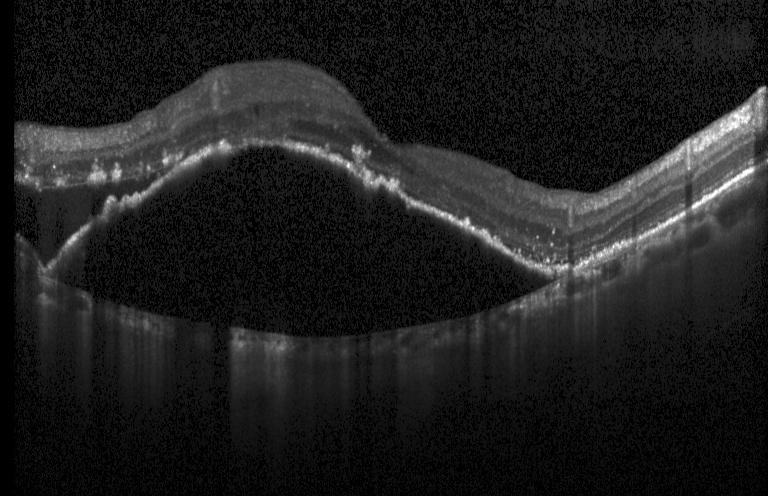
Optical coherence tomography B-scan. Acquired on a Heidelberg Spectralis.
Dx: CNV.